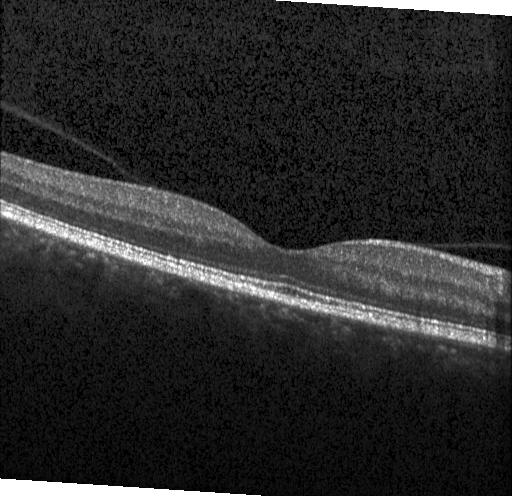 OCT scan showing no CNV, no DME, and no drusen.